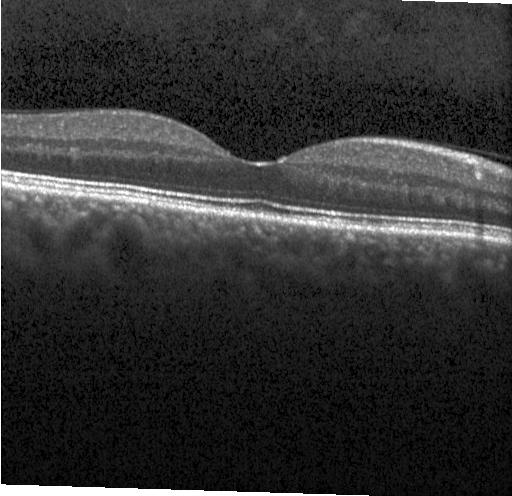

OCT line scan — Impression: no evidence of CNV, DME, or drusen.